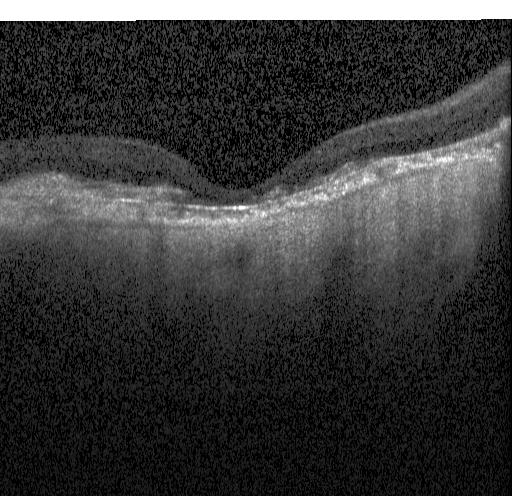

This B-scan demonstrates a choroidal neovascular membrane.